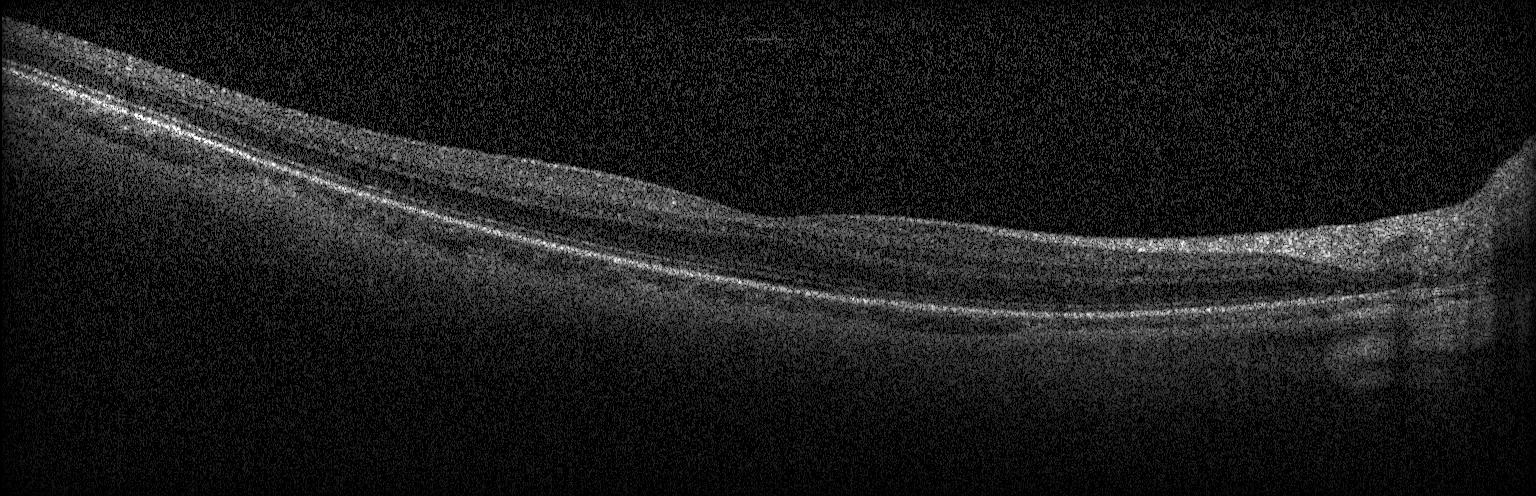

Spectral-domain OCT B-scan: no evidence of choroidal neovascularization, diabetic macular edema, or drusen.